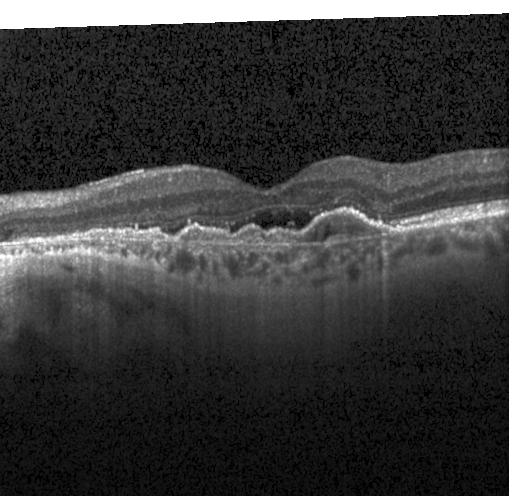
Instrument: Heidelberg Spectralis. Optical coherence tomography B-scan. SD-OCT.
Finding: a choroidal neovascular membrane.